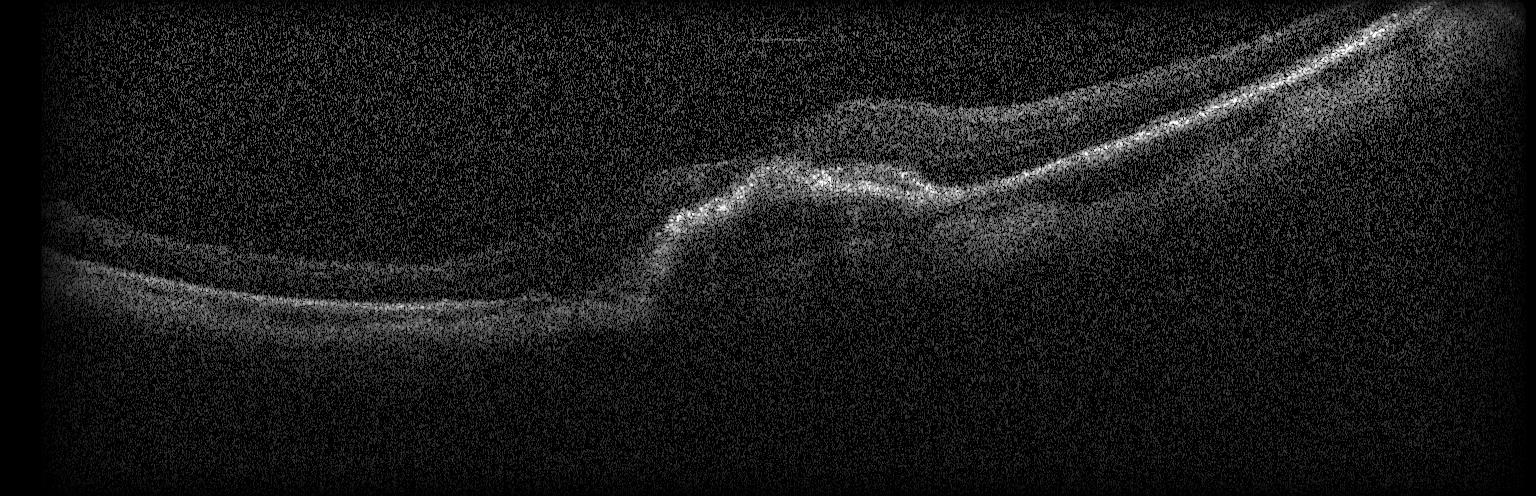
This B-scan demonstrates choroidal neovascularization (CNV).